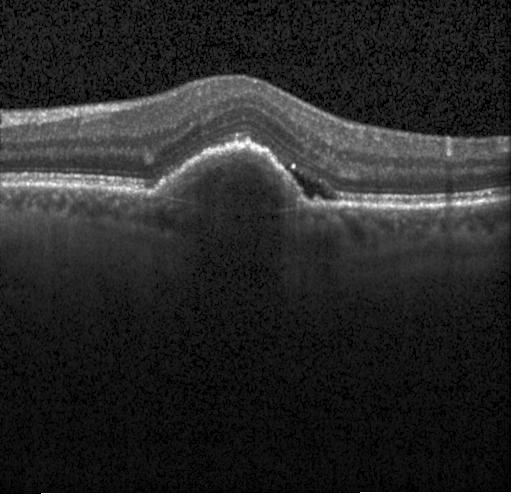

Centered on the fovea; retinal OCT cross-section; instrument: Heidelberg Spectralis; spectral-domain optical coherence tomography.
Diagnosis: CNV.